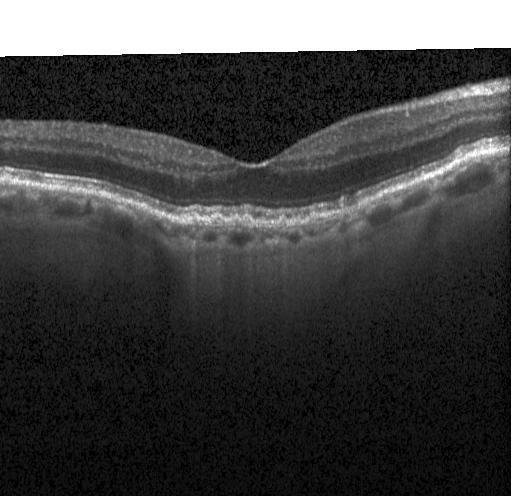 Spectral-domain optical coherence tomography · retinal OCT B-scan.
Diagnosis: sub-RPE drusenoid deposits.